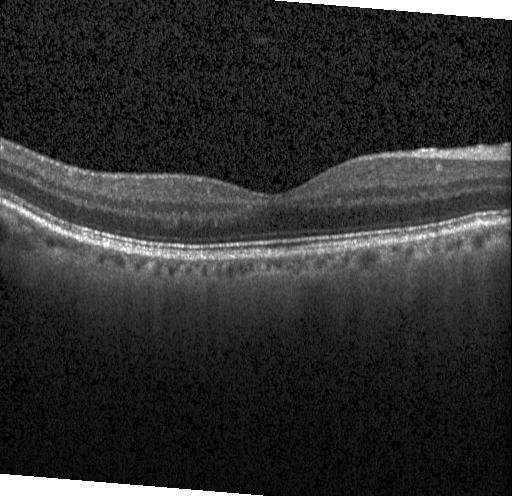
Impression: no CNV, DME, or drusen.